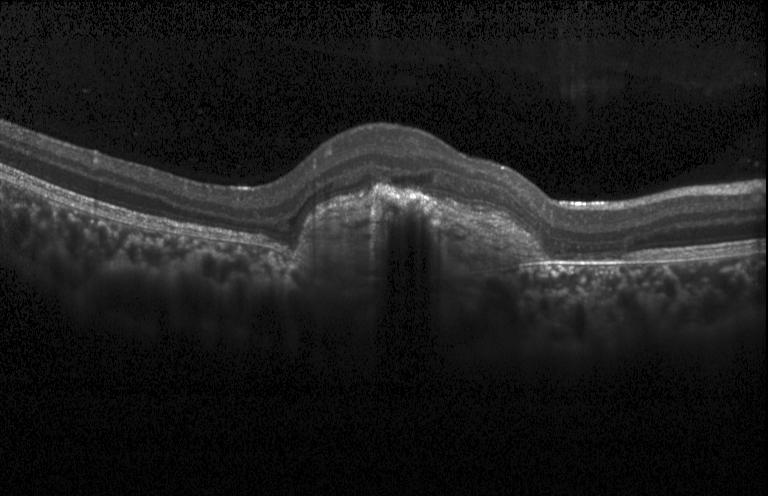
Through the macula · optical coherence tomography B-scan · Heidelberg Spectralis OCT system — Impression: a choroidal neovascular membrane.